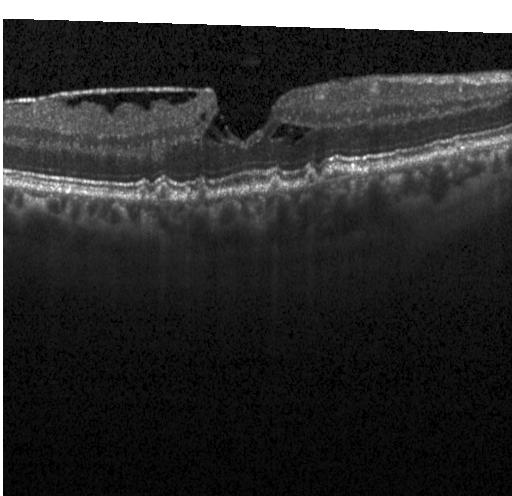 OCT line scan; fovea-centered; instrument: Heidelberg Spectralis; SD-OCT. Finding: multiple drusen.